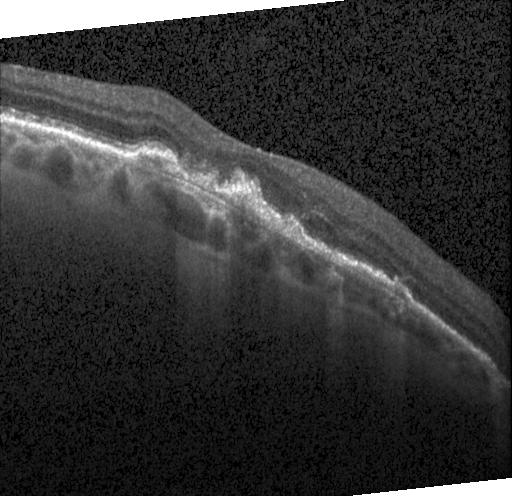
Assessment: CNV.